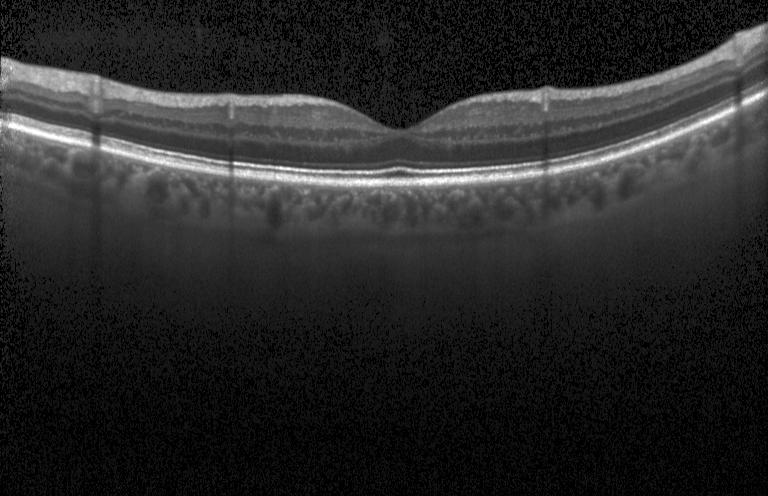

Retinal OCT cross-section
Macular OCT: no evidence of choroidal neovascularization, diabetic macular edema, or drusen.